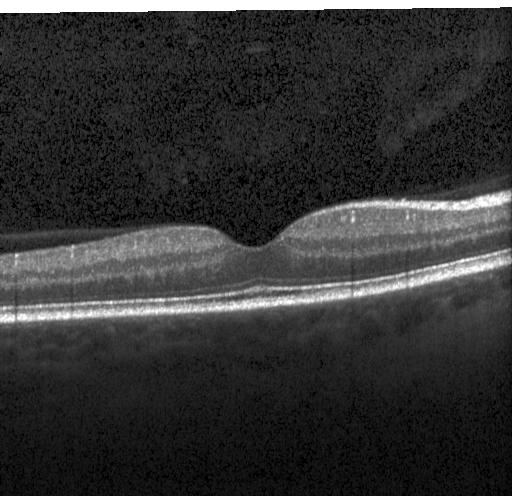

OCT finding: no evidence of CNV, DME, or drusen.